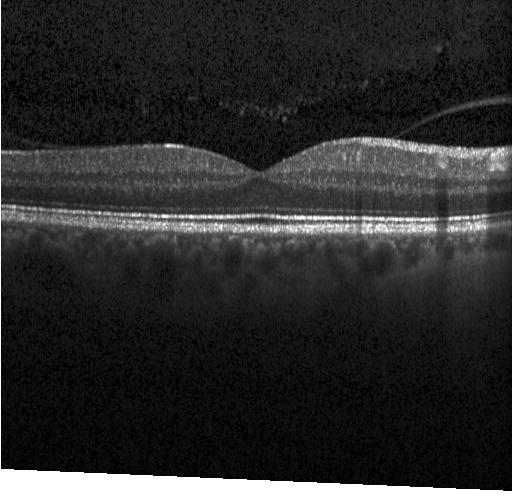 The scan shows no choroidal neovascularization, no diabetic macular edema, and no drusen.